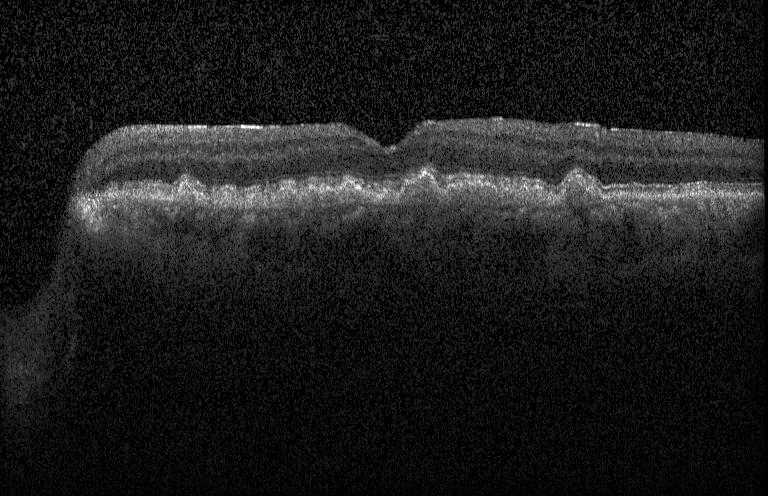 Diagnosis: choroidal neovascularization.